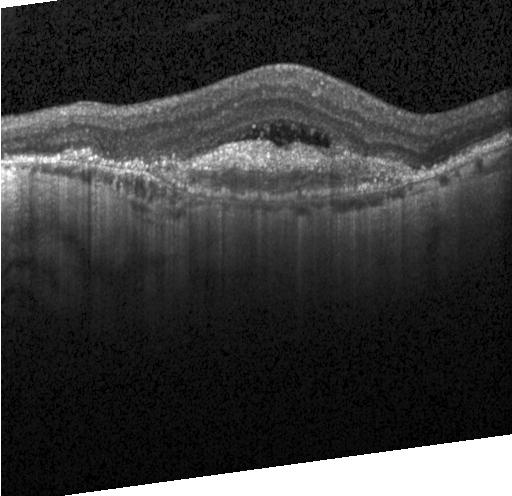
SD-OCT · fovea-centered · retinal OCT cross-section · instrument: Heidelberg Spectralis. The scan shows choroidal neovascularization.